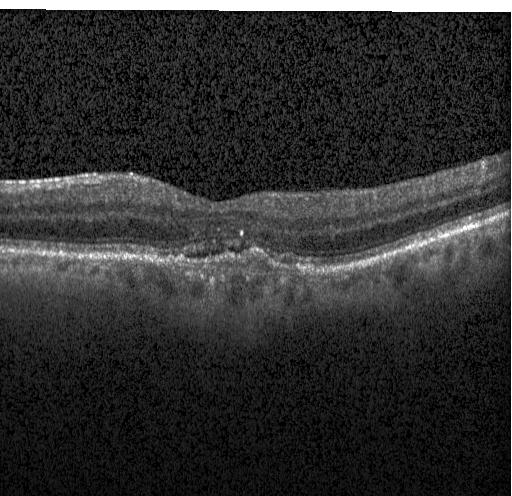 Diagnosis: a choroidal neovascular membrane.